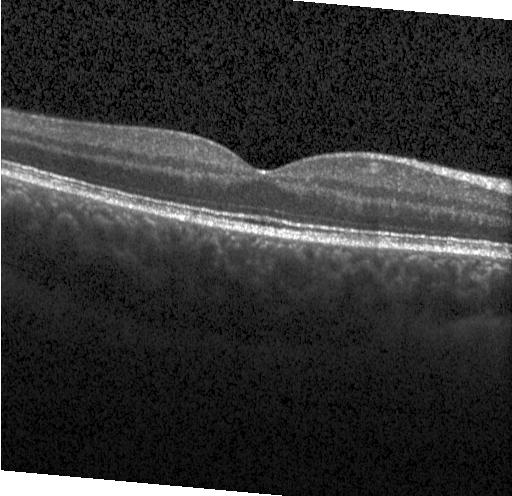
OCT line scan. Fovea-centered. Spectral-domain OCT. Impression: no choroidal neovascularization, diabetic macular edema, or drusen.